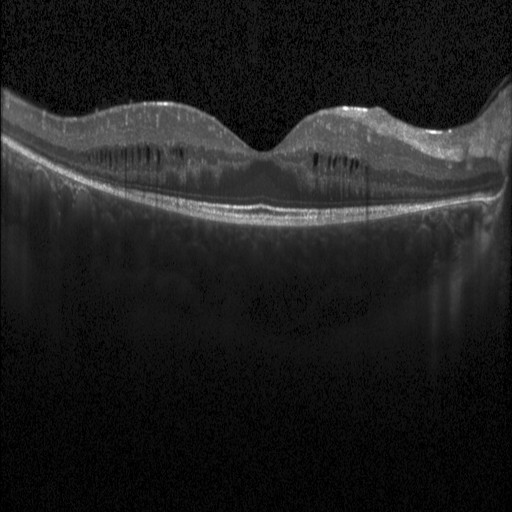 Dx: diabetic macular edema (DME).